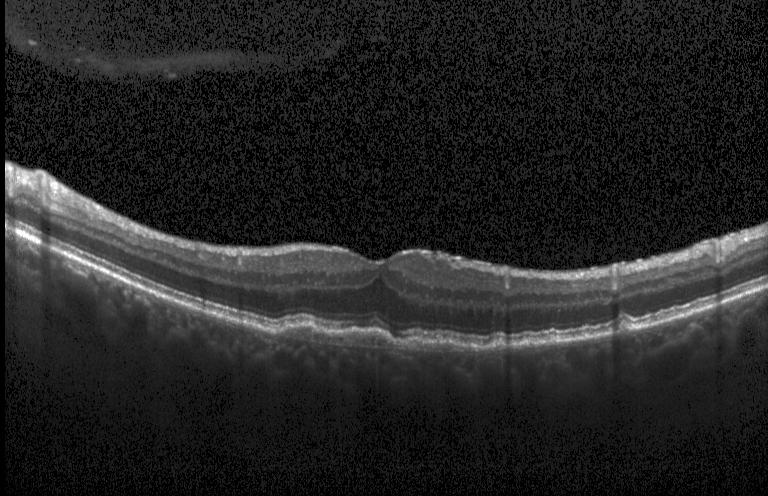 Impression: a choroidal neovascular membrane.